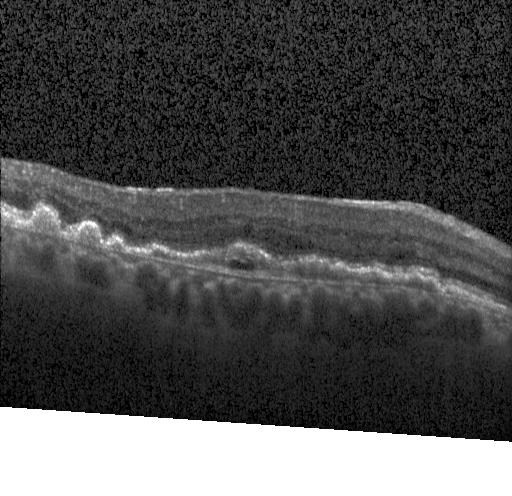 Heidelberg Spectralis. Centered on the fovea. Retinal OCT B-scan
This B-scan demonstrates choroidal neovascularization (CNV).